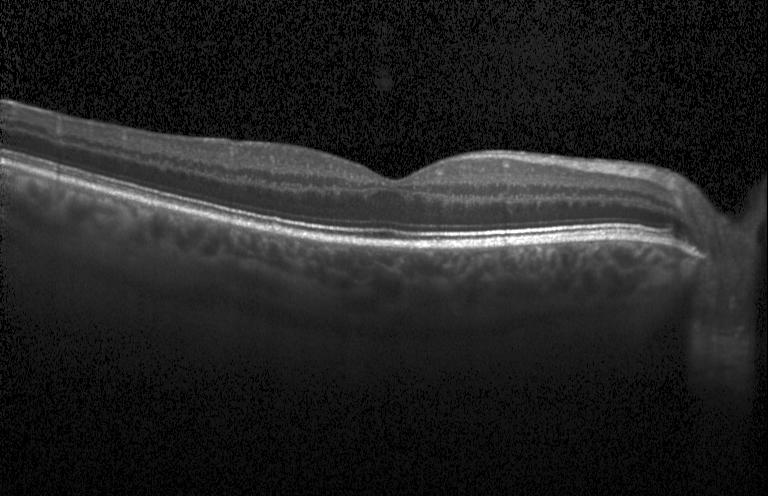

Retinal OCT cross-section · through the macula
Assessment: no choroidal neovascularization, no diabetic macular edema, and no drusen.